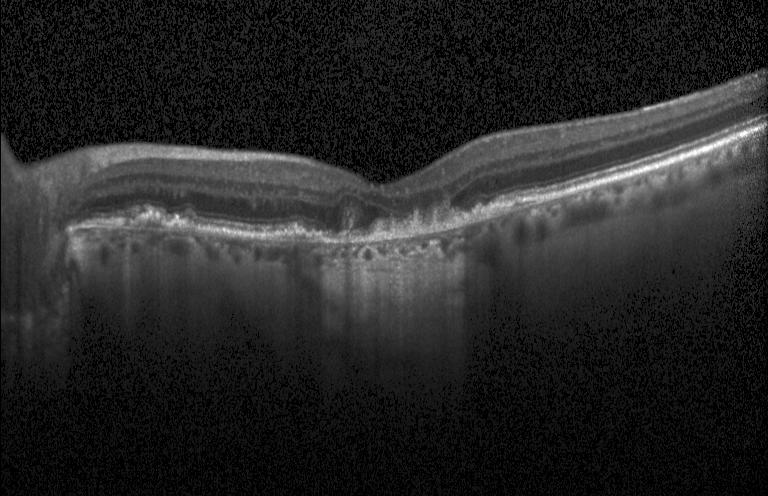
Heidelberg Spectralis; optical coherence tomography B-scan; spectral-domain OCT; centered on the fovea
Dx: CNV.